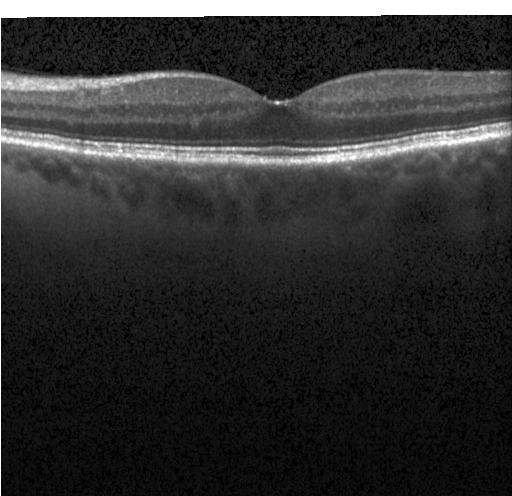
Spectral-domain optical coherence tomography. OCT B-scan.
Impression: no CNV, DME, or drusen.